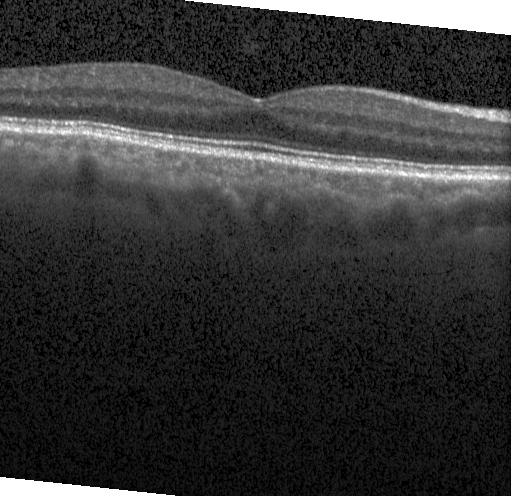 Optical coherence tomography scan, spectral-domain OCT, acquired on a Heidelberg Spectralis — Impression: neither choroidal neovascularization, diabetic macular edema, nor drusen.